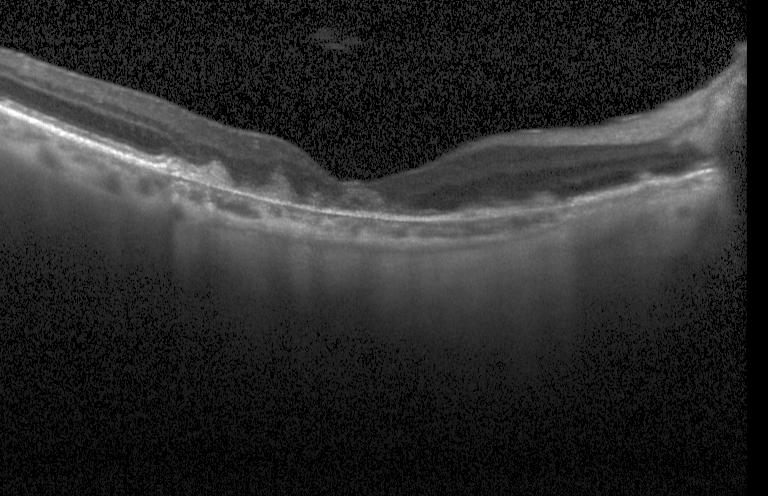

SD-OCT, optical coherence tomography scan, centered on the fovea, instrument: Heidelberg Spectralis — Impression: a choroidal neovascular membrane.